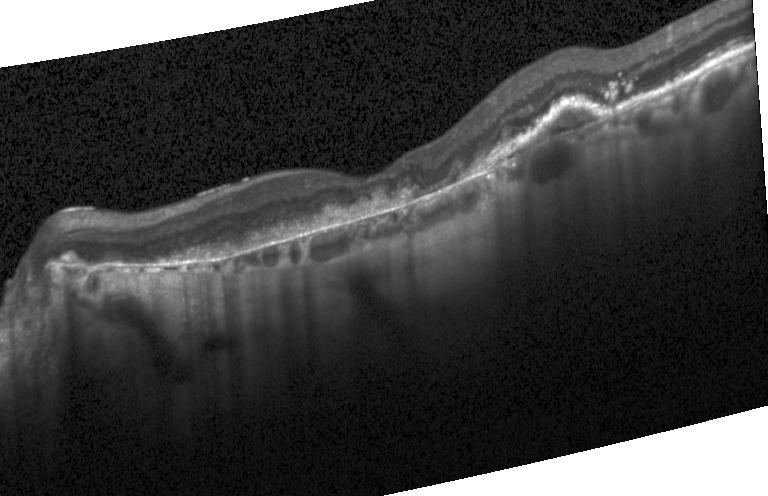 Spectral-domain OCT B-scan: CNV.